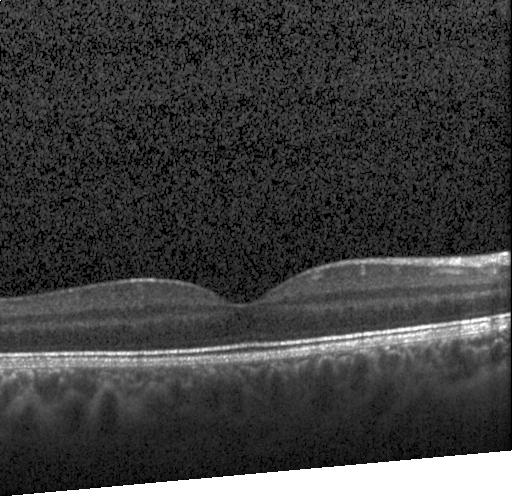 Acquired on a Heidelberg Spectralis · spectral-domain OCT · fovea-centered · retinal OCT B-scan
No CNV, DME, or drusen.